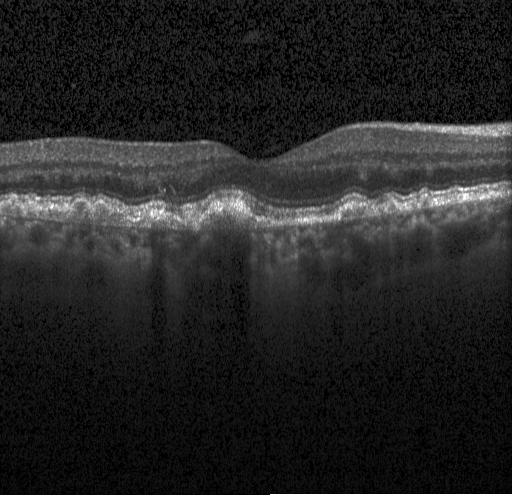

Through the macula. Retinal OCT cross-section. The scan shows sub-RPE drusenoid deposits.